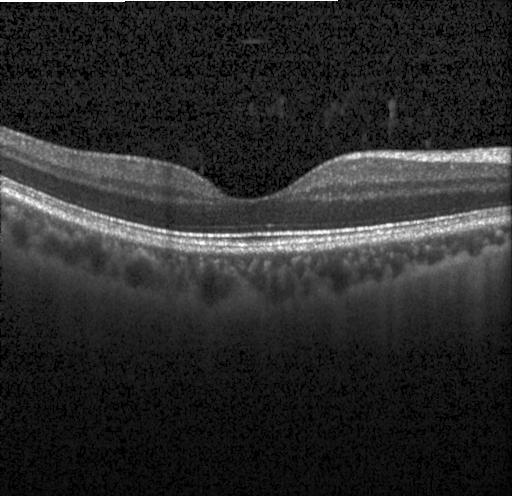 OCT scan showing no CNV, no DME, and no drusen.